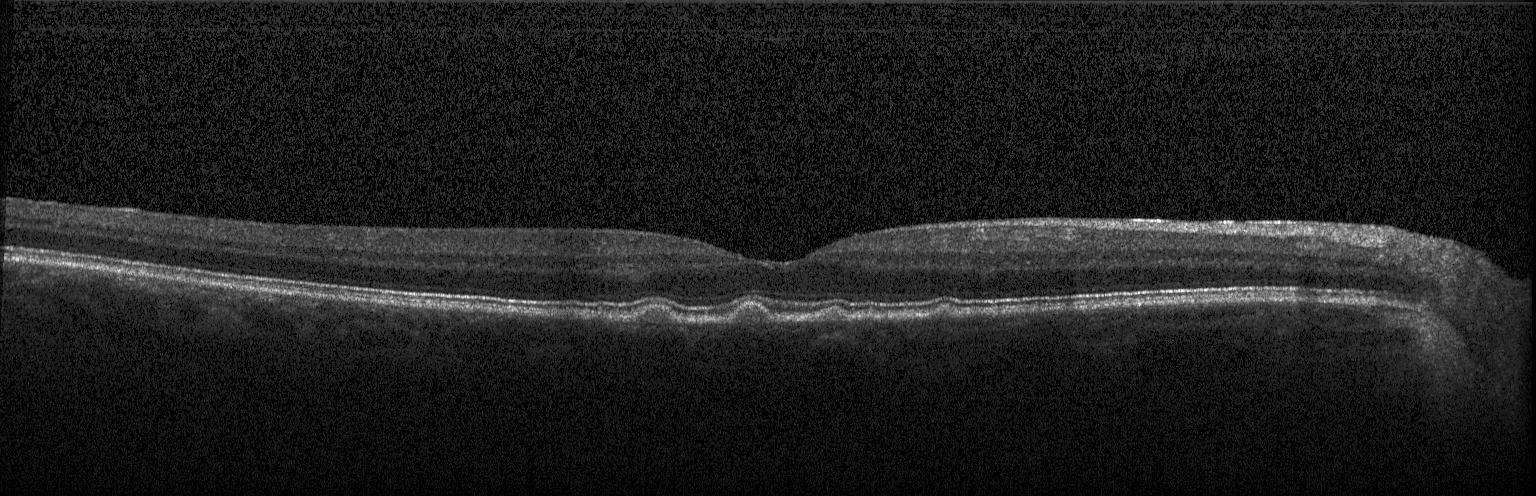

Retinal OCT cross-section. Diagnosis: multiple drusen.